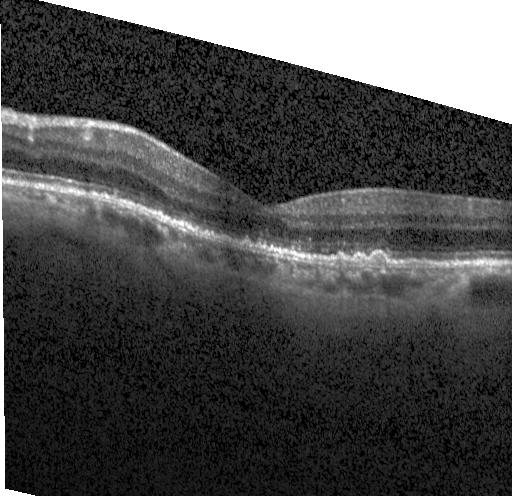 OCT B-scan
Multiple drusen.